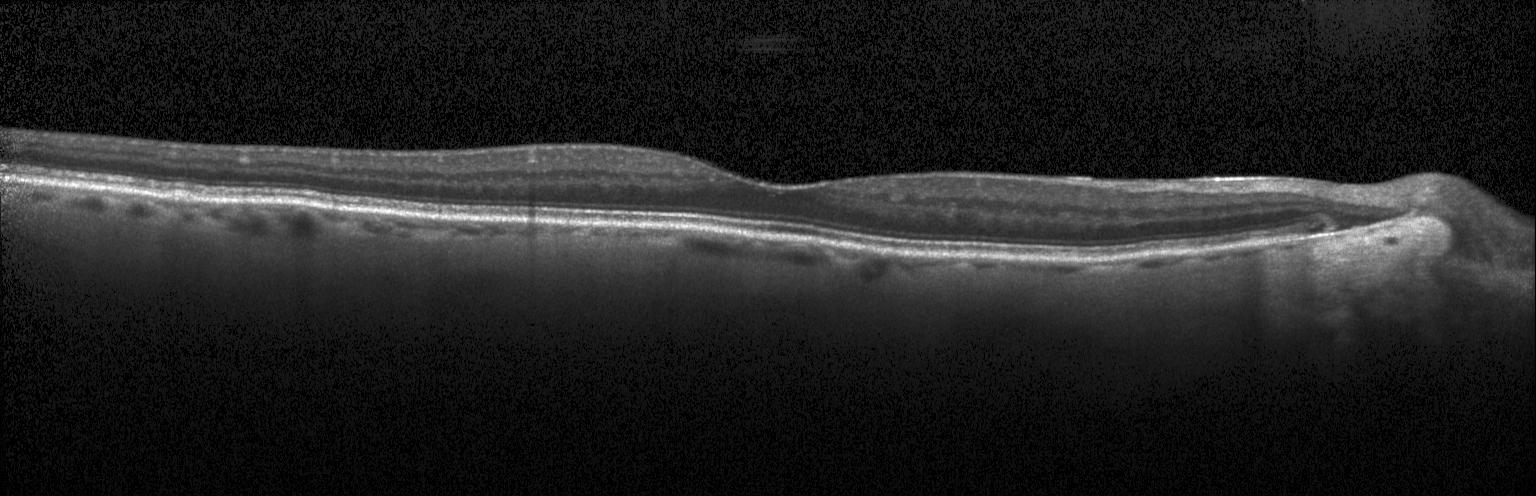
OCT B-scan showing no evidence of CNV, DME, or drusen.